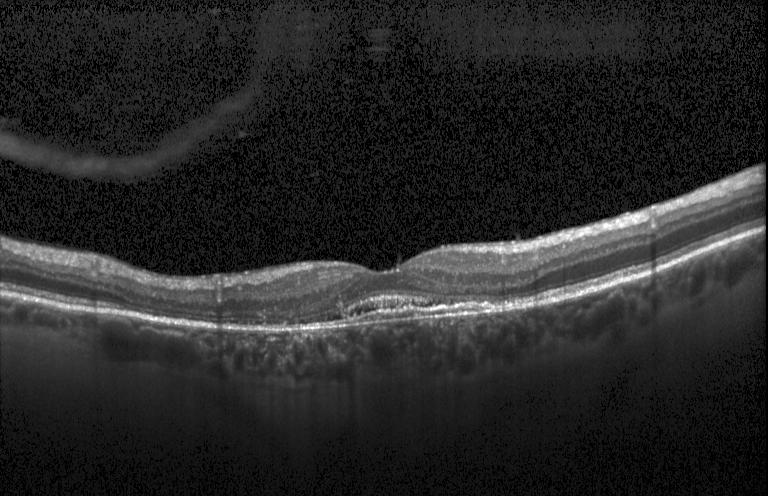

Dx: choroidal neovascularization.